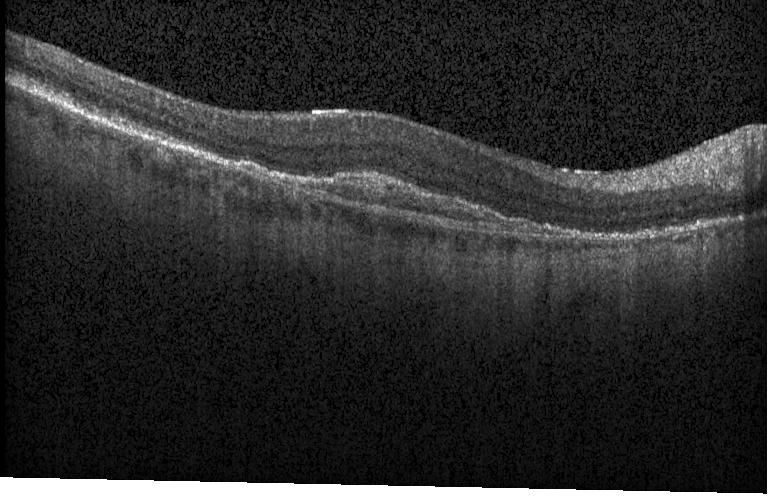

Through the macula. Optical coherence tomography scan. Instrument: Heidelberg Spectralis. Dx: a choroidal neovascular membrane.